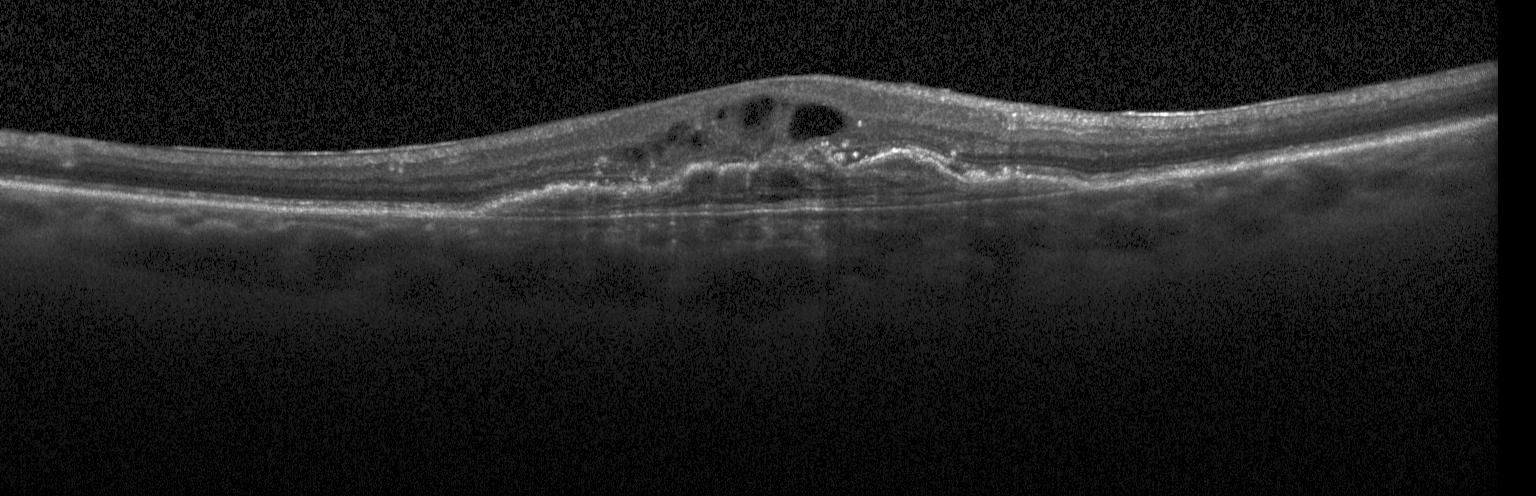

The scan shows CNV.